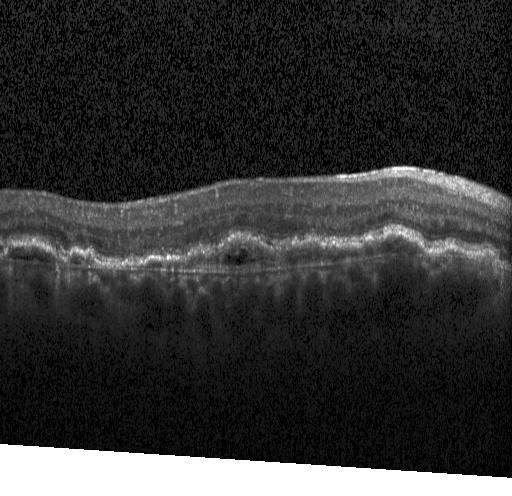 Centered on the fovea; instrument: Heidelberg Spectralis; retinal OCT B-scan; spectral-domain optical coherence tomography. Assessment: a choroidal neovascular membrane.